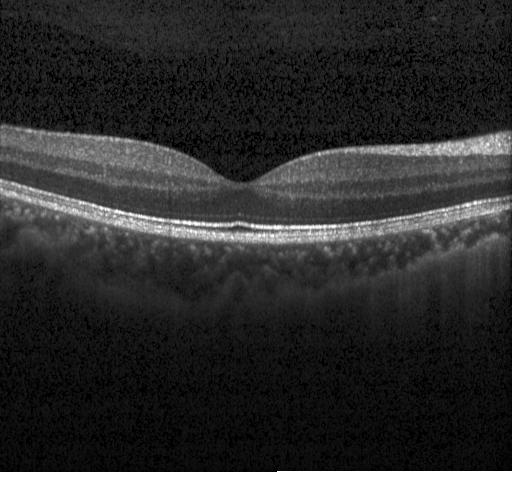

Retinal OCT B-scan.
Finding: no choroidal neovascularization, diabetic macular edema, or drusen.